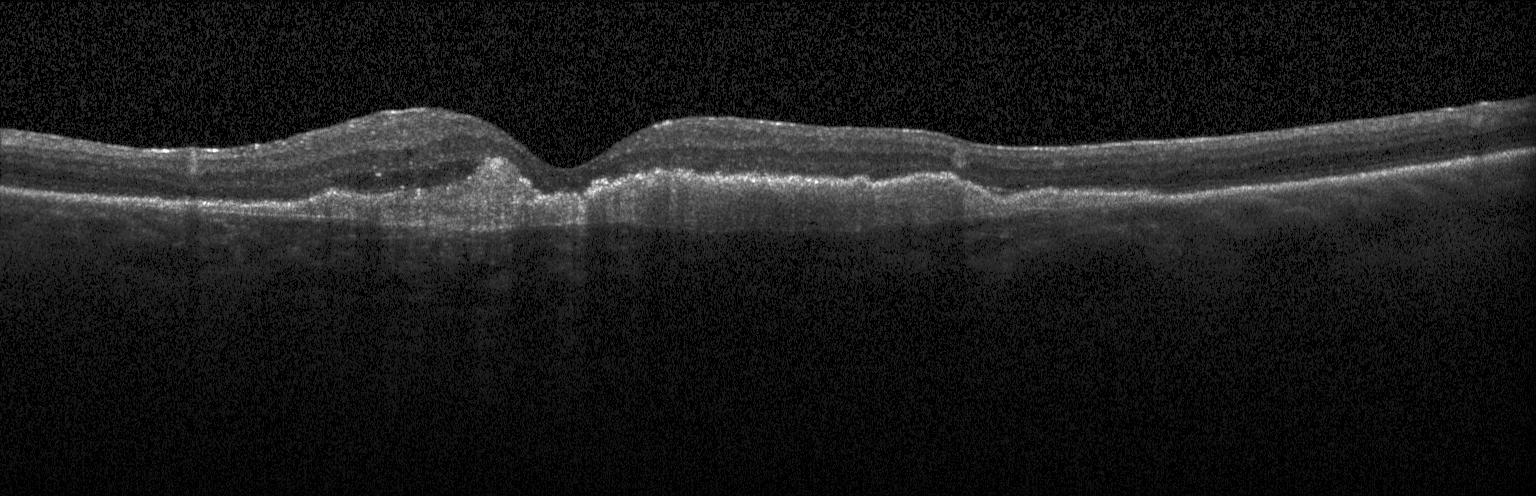
Retinal OCT B-scan
Assessment: choroidal neovascularization (CNV).